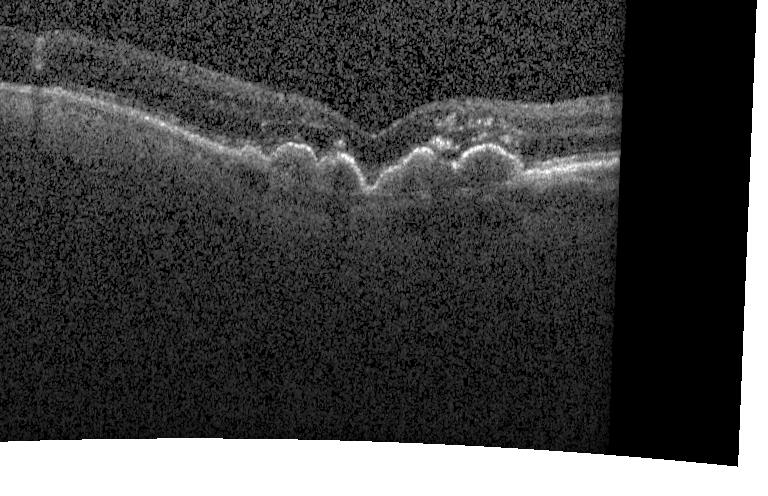

Heidelberg Spectralis OCT system; horizontal scan through the fovea; OCT B-scan. Impression: a choroidal neovascular membrane.